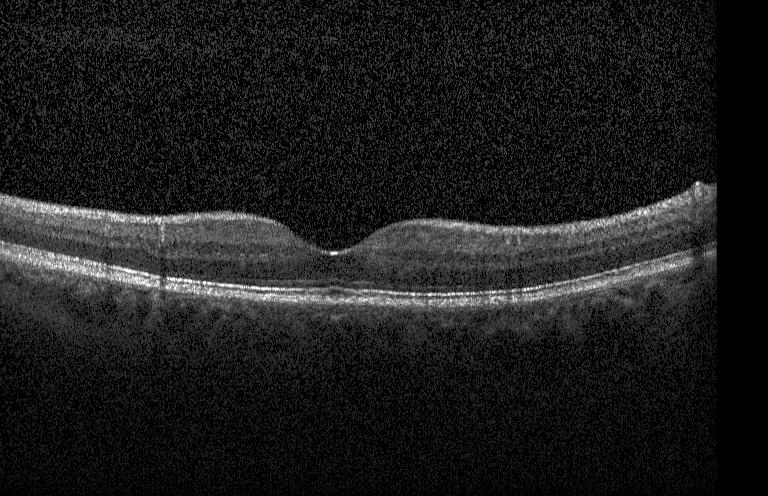
Optical coherence tomography scan — Finding: neither choroidal neovascularization, diabetic macular edema, nor drusen.